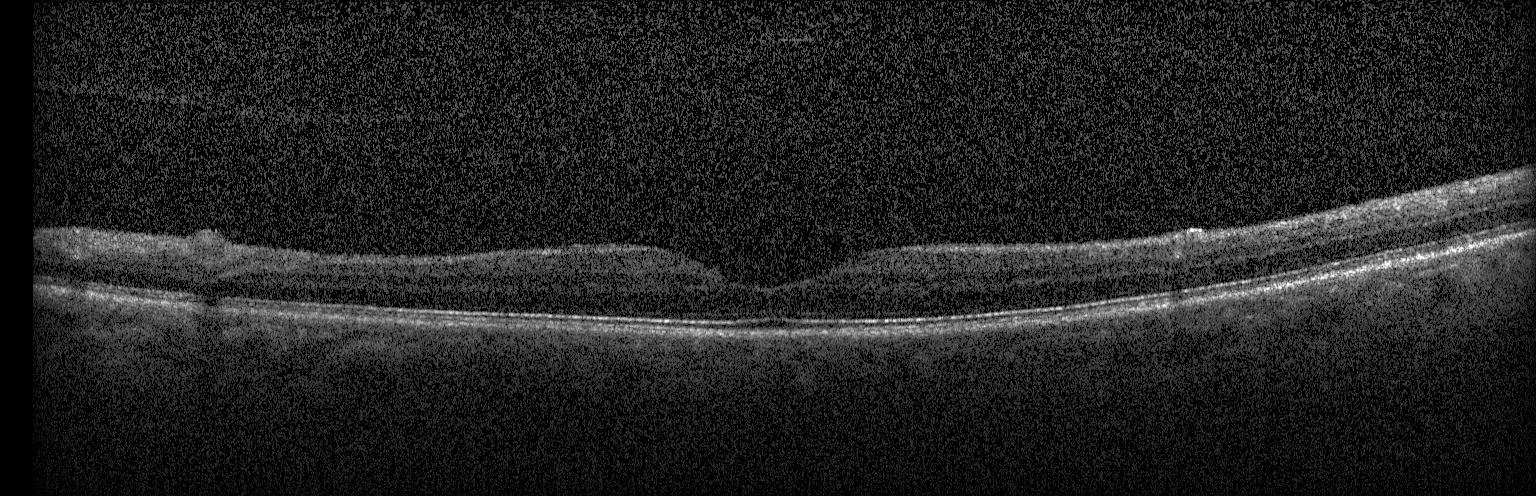

Centered on the fovea · OCT line scan. Impression: no CNV, no DME, and no drusen.